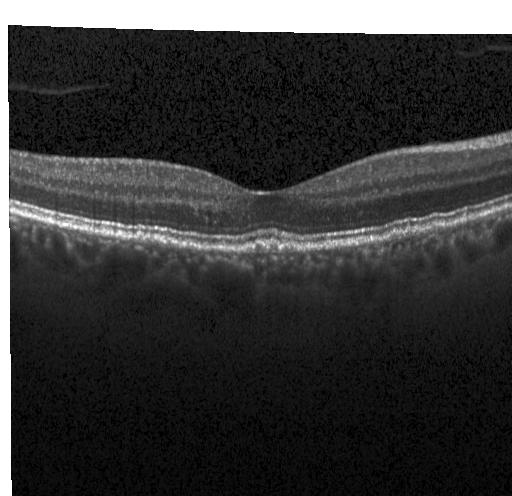

Impression: drusen.